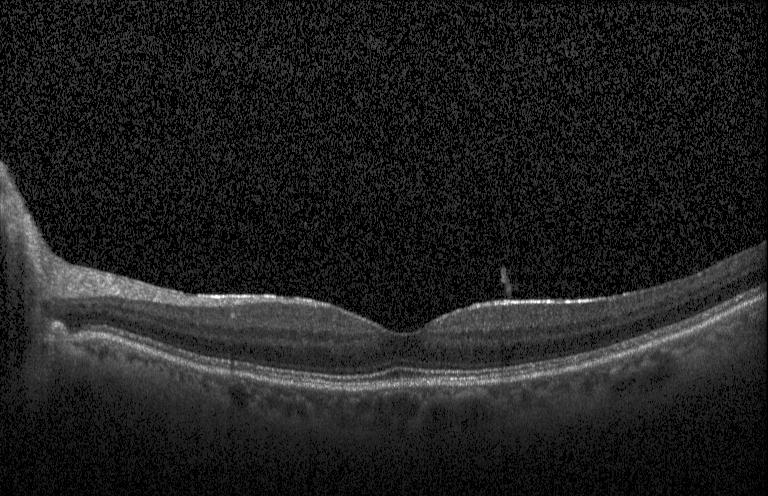 Through the macula. Spectral-domain optical coherence tomography. Optical coherence tomography B-scan — Impression: no CNV, no DME, and no drusen.